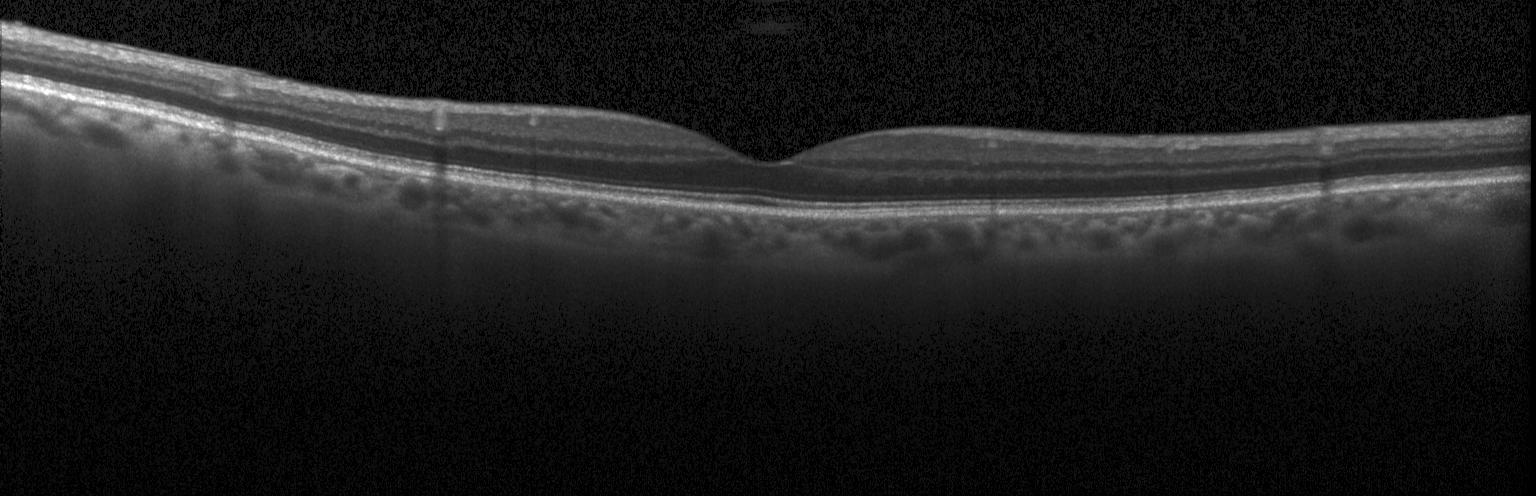

Diagnosis: no CNV, DME, or drusen.